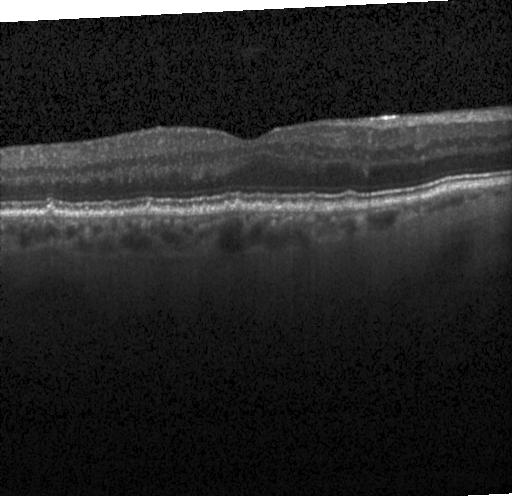 Instrument: Heidelberg Spectralis, SD-OCT, optical coherence tomography B-scan, centered on the fovea
Diagnosis: sub-RPE drusenoid deposits.